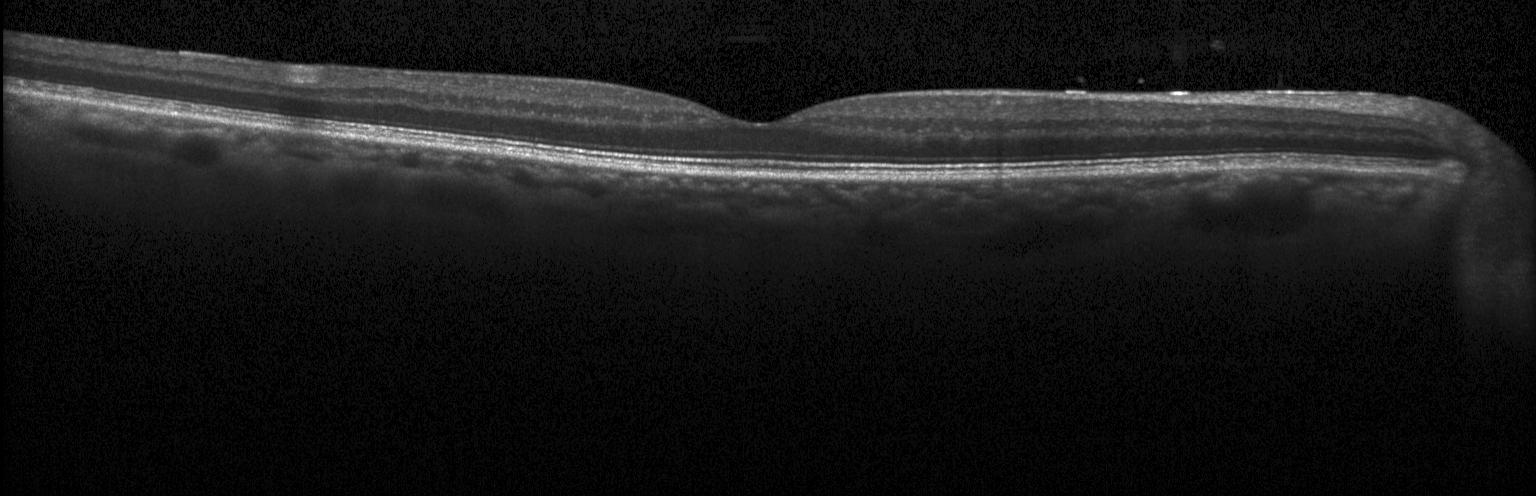 OCT line scan.
Finding: no choroidal neovascularization, no diabetic macular edema, and no drusen.